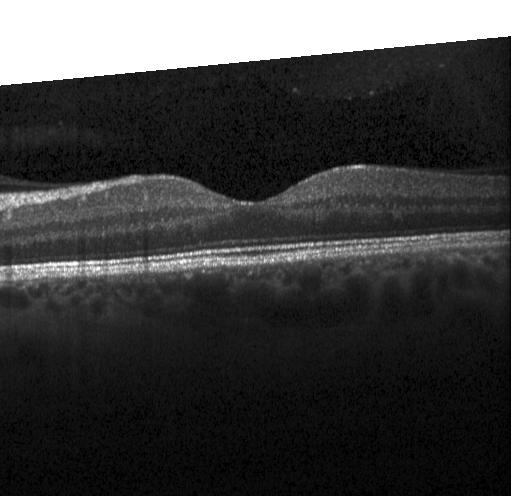

SD-OCT; OCT line scan
Assessment: no CNV, DME, or drusen.